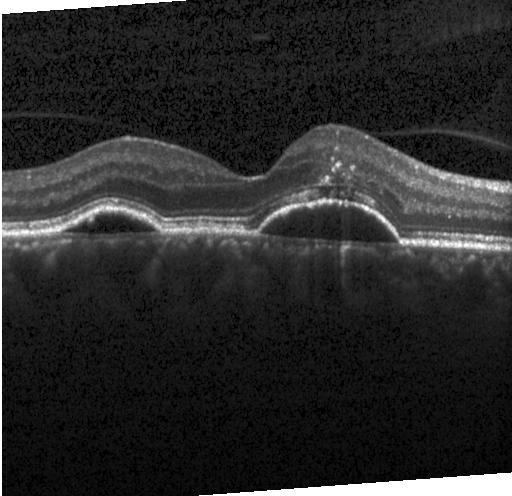
Spectral-domain OCT; optical coherence tomography scan — Impression: a choroidal neovascular membrane.